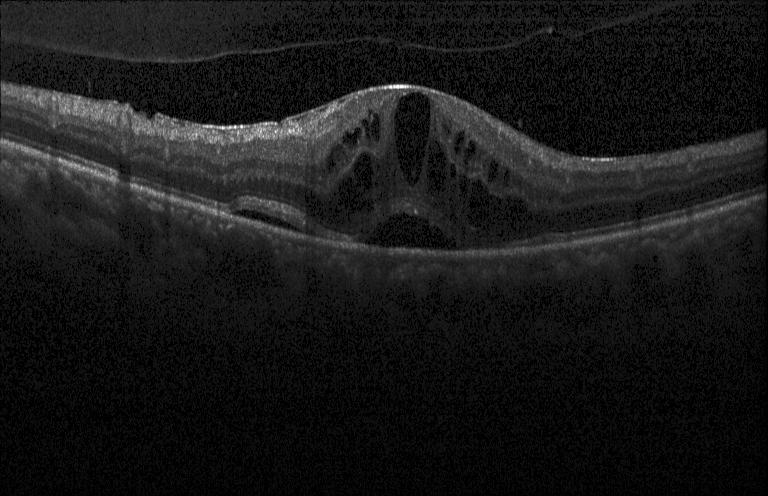
Optical coherence tomography B-scan. The scan shows diabetic macular edema (DME).